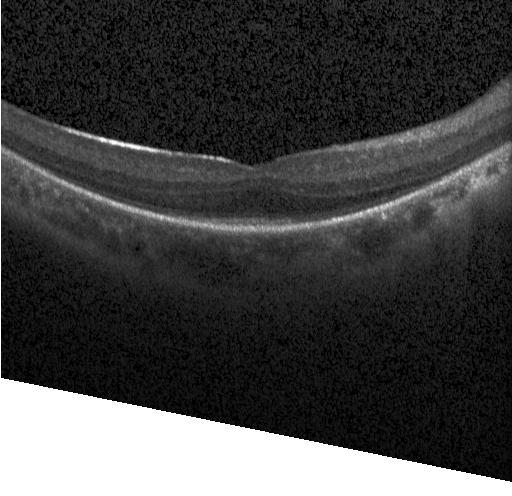

Finding: neither choroidal neovascularization, diabetic macular edema, nor drusen.